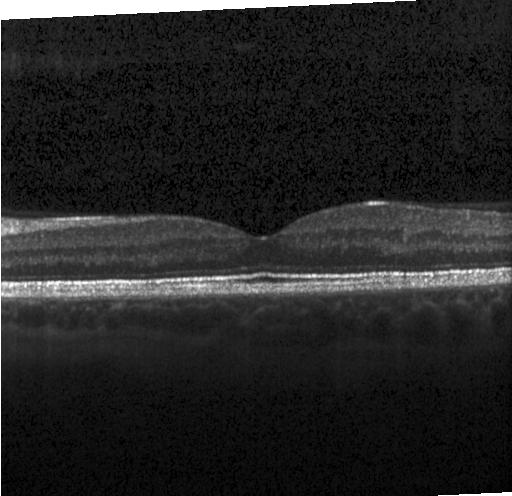

OCT finding: no evidence of choroidal neovascularization, diabetic macular edema, or drusen.